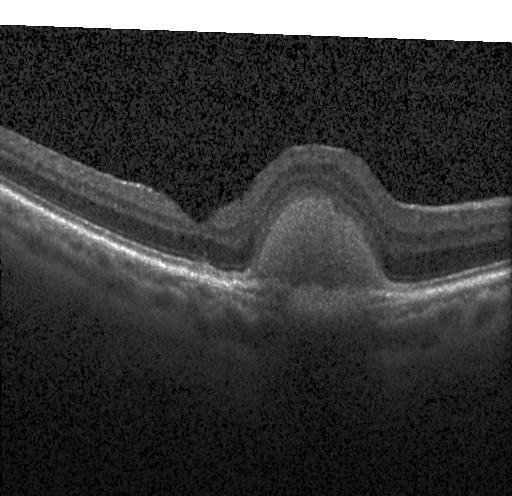 OCT B-scan, SD-OCT, acquired on a Heidelberg Spectralis — Choroidal neovascularization.